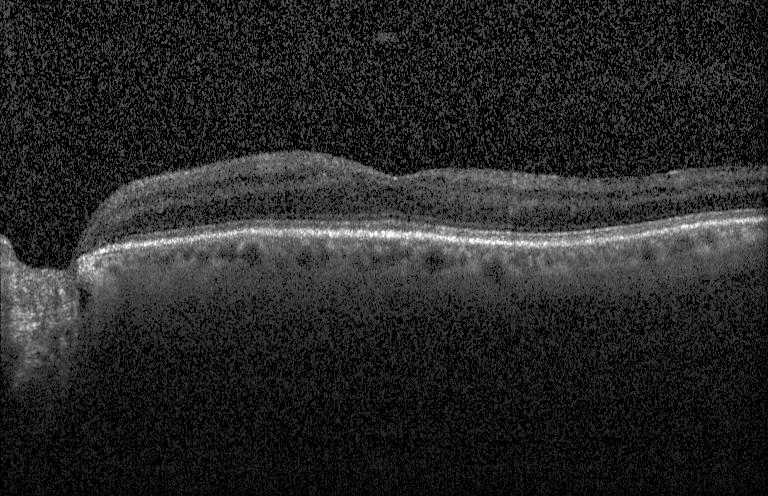

OCT B-scan; Heidelberg Spectralis; SD-OCT; macular scan
Impression: no choroidal neovascularization, no diabetic macular edema, and no drusen.